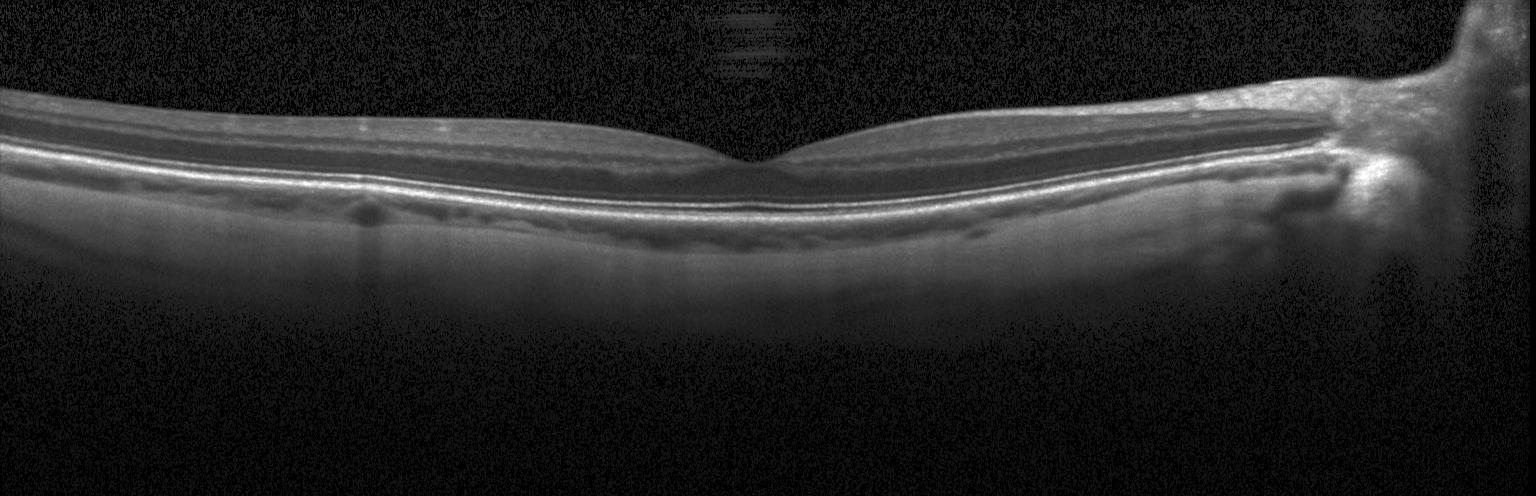

Retinal OCT cross-section. Spectral-domain optical coherence tomography. Acquired on a Heidelberg Spectralis. Fovea-centered.
Impression: no CNV, no DME, and no drusen.